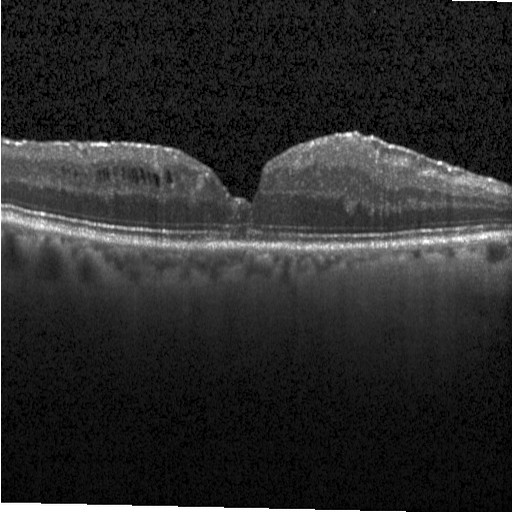

Through the macula; instrument: Heidelberg Spectralis; spectral-domain OCT; OCT line scan.
Diagnosis: diabetic macular edema.